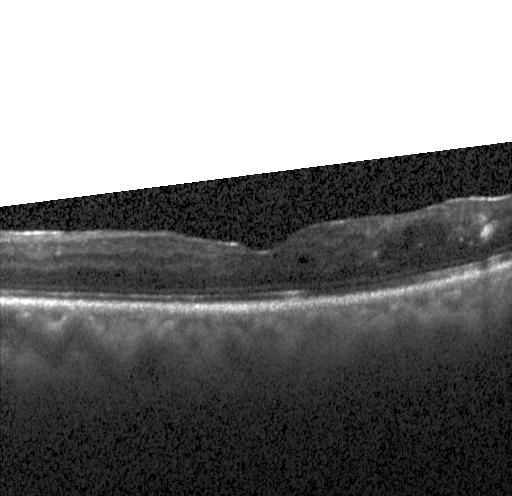

OCT B-scan. Spectral-domain OCT. Macular scan. Instrument: Heidelberg Spectralis. Macular OCT: diabetic macular edema (DME).